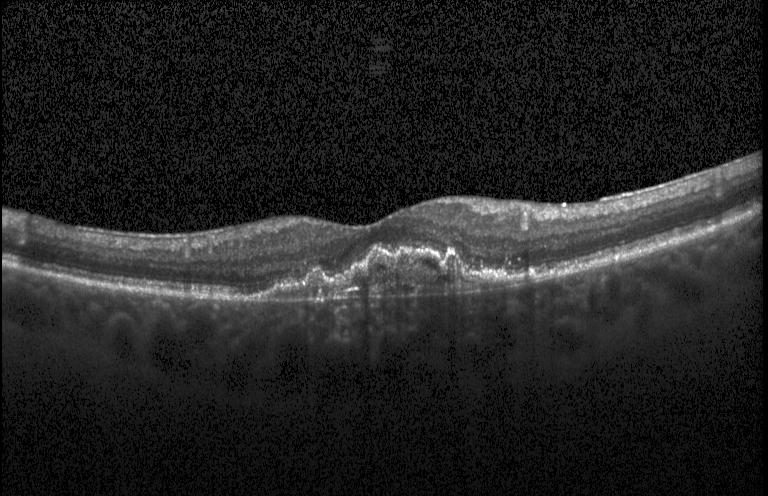

Dx: a choroidal neovascular membrane.